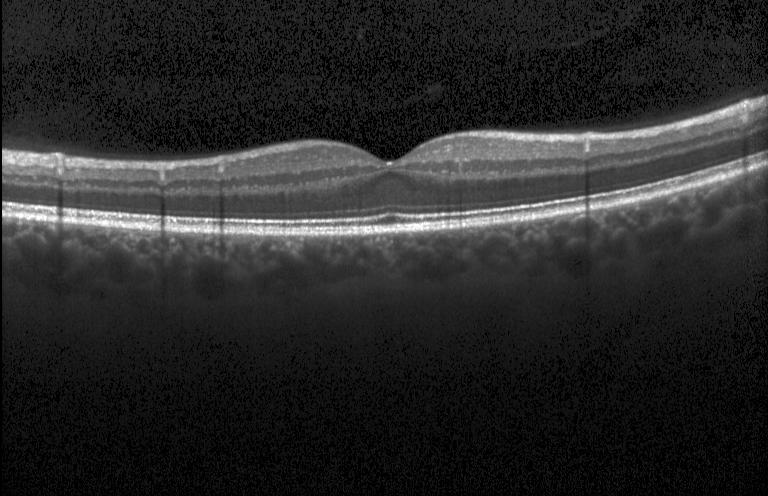

Spectral-domain OCT. Optical coherence tomography scan. Horizontal scan through the fovea. Heidelberg Spectralis
OCT finding: no evidence of CNV, DME, or drusen.